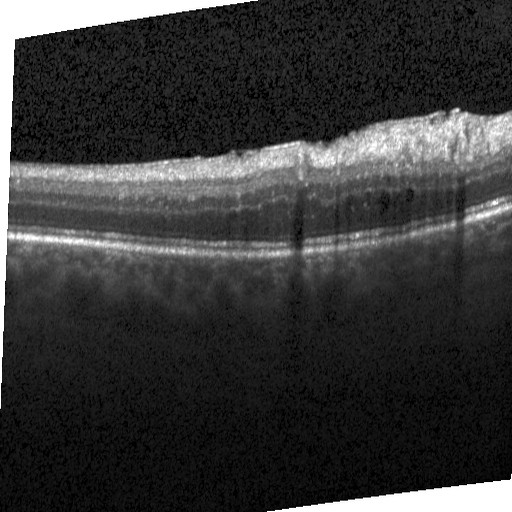 OCT B-scan showing diabetic macular edema (DME).